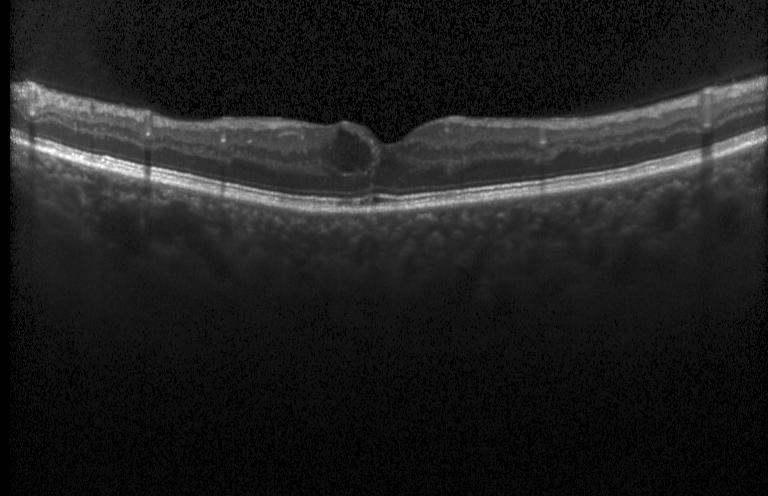

Retinal OCT cross-section; Heidelberg Spectralis; macular scan; SD-OCT.
Diagnosis: diabetic macular edema (DME).